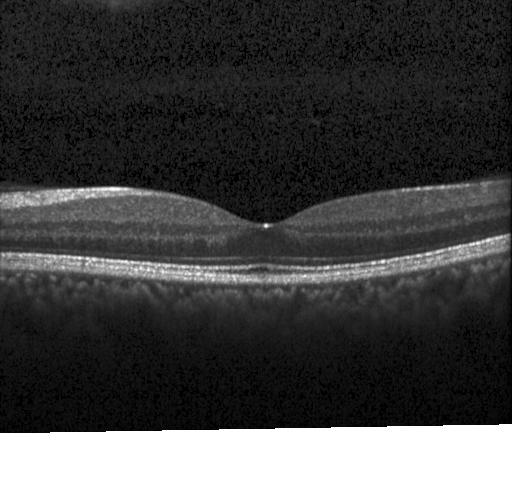
Finding: no choroidal neovascularization, no diabetic macular edema, and no drusen.